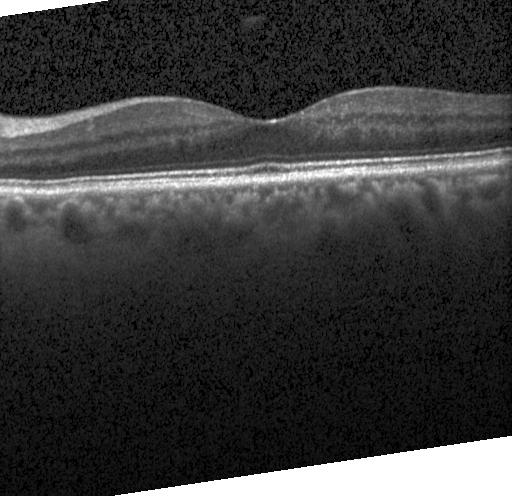

Optical coherence tomography scan. Instrument: Heidelberg Spectralis — Diagnosis: no choroidal neovascularization, diabetic macular edema, or drusen.